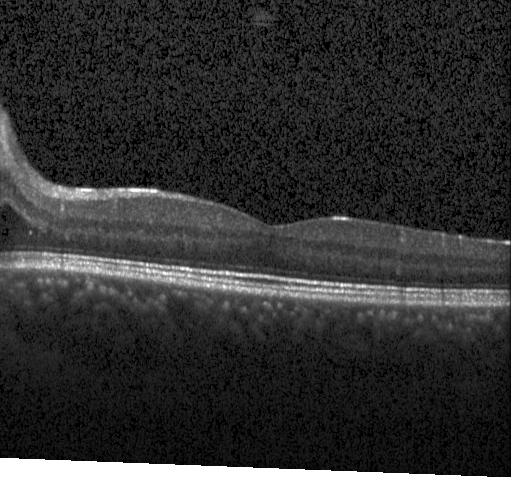
Assessment: no evidence of choroidal neovascularization, diabetic macular edema, or drusen.